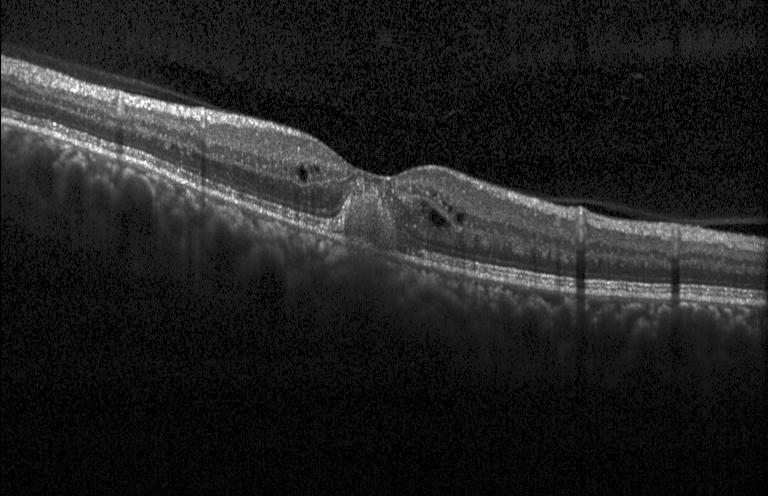

OCT B-scan.
This B-scan demonstrates a choroidal neovascular membrane.